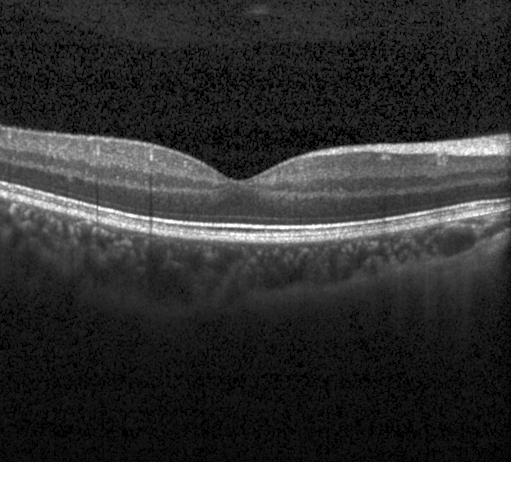
Optical coherence tomography scan. Through the macula. Spectral-domain optical coherence tomography — OCT finding: no CNV, no DME, and no drusen.